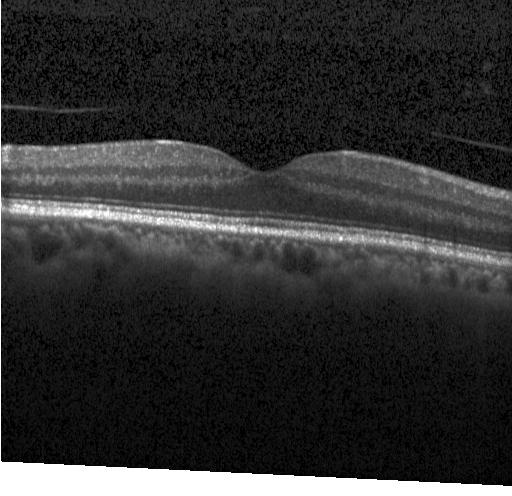
Horizontal scan through the fovea · optical coherence tomography B-scan · SD-OCT.
Assessment: no CNV, no DME, and no drusen.